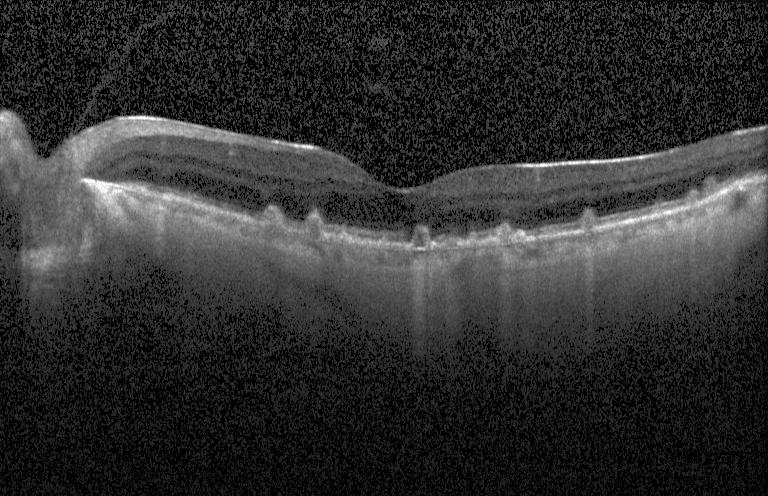 OCT B-scan. Centered on the fovea
Finding: drusen.